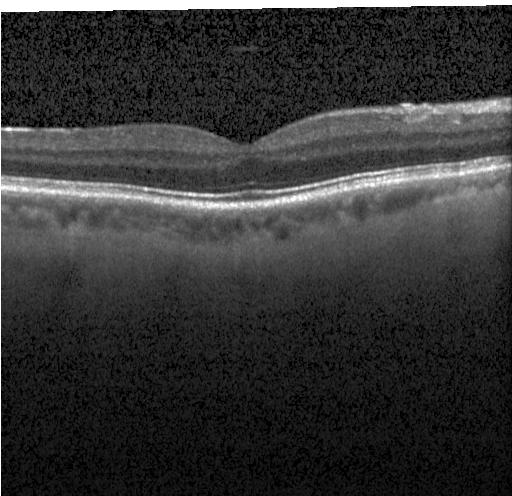

Macular scan, retinal OCT B-scan. Dx: no CNV, DME, or drusen.